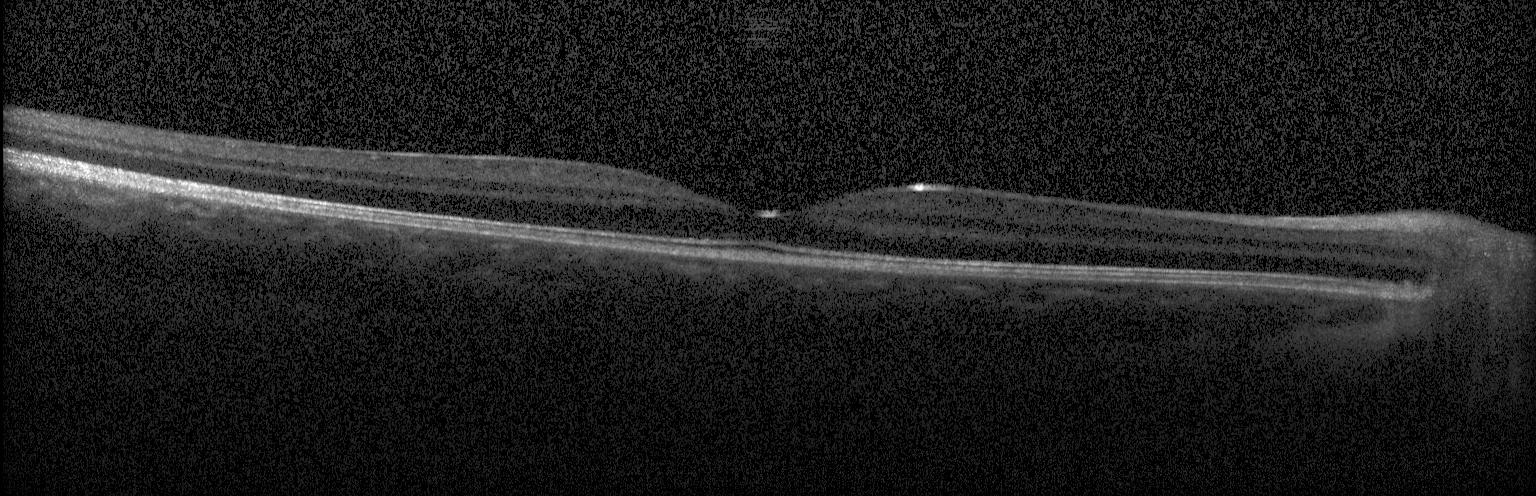 Impression: no evidence of choroidal neovascularization, diabetic macular edema, or drusen.